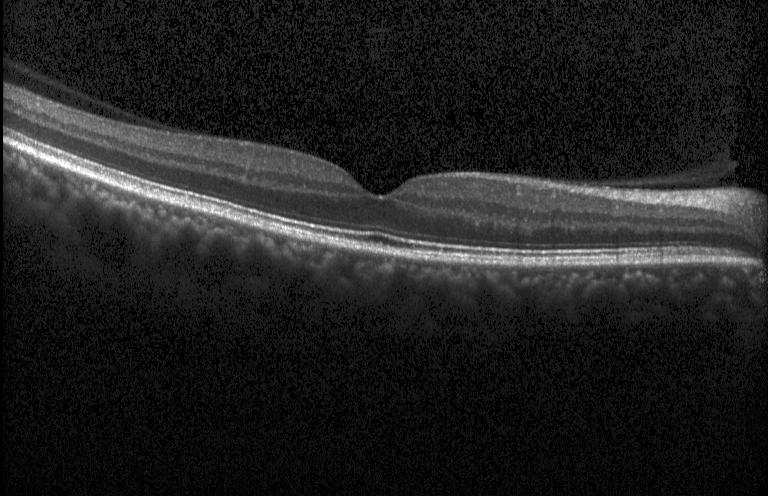

OCT B-scan — Impression: no choroidal neovascularization, no diabetic macular edema, and no drusen.